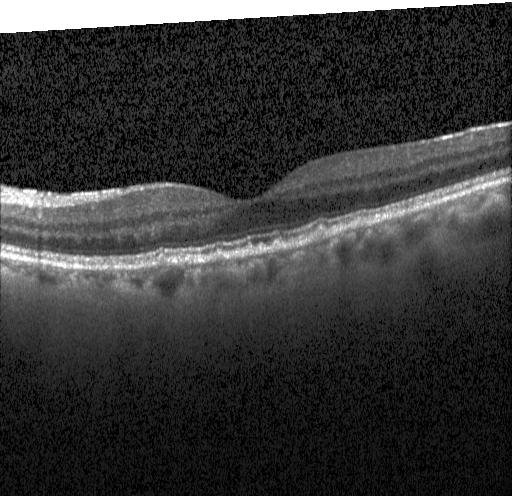 Horizontal scan through the fovea, instrument: Heidelberg Spectralis, OCT B-scan, spectral-domain OCT — The scan shows drusen.